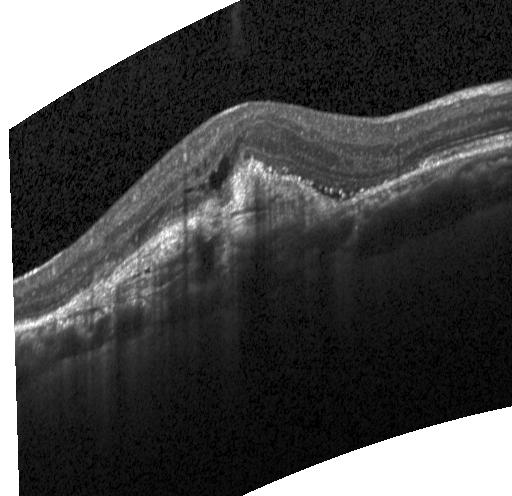 Retinal OCT cross-section; macular scan — Diagnosis: a choroidal neovascular membrane.